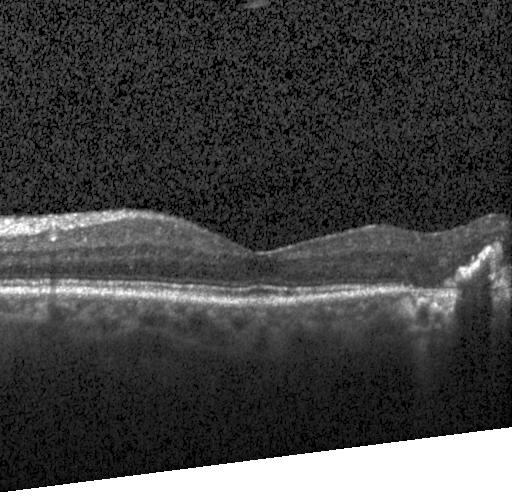

Retinal OCT cross-section showing choroidal neovascularization.